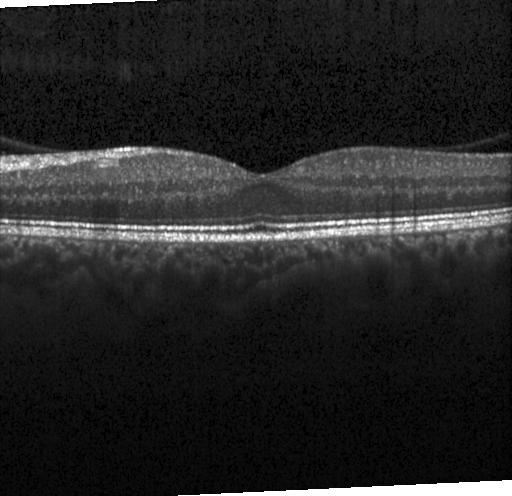

SD-OCT; retinal OCT cross-section; instrument: Heidelberg Spectralis. Impression: neither choroidal neovascularization, diabetic macular edema, nor drusen.